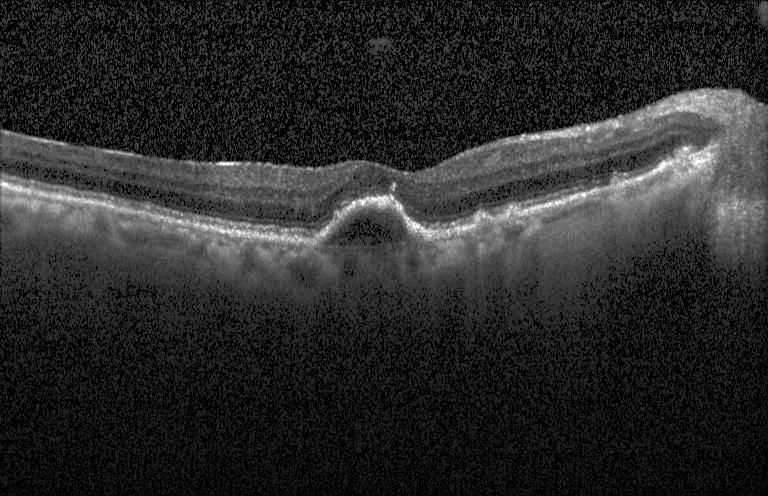

Retinal OCT cross-section showing a choroidal neovascular membrane.